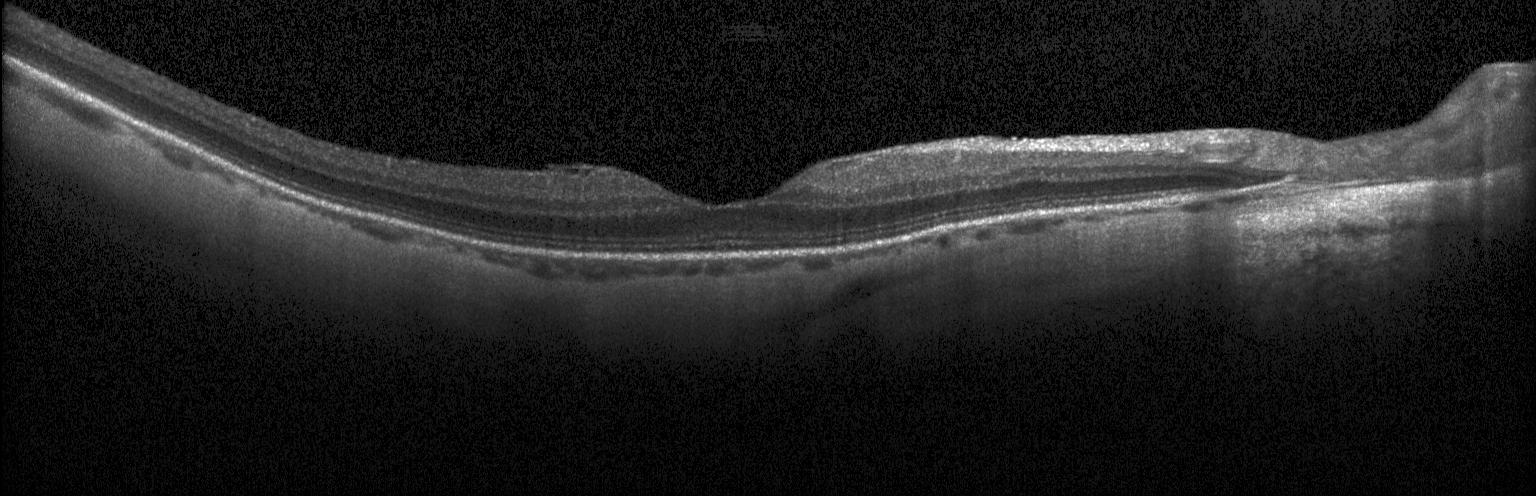
Fovea-centered · spectral-domain OCT · OCT B-scan. OCT finding: no evidence of choroidal neovascularization, diabetic macular edema, or drusen.